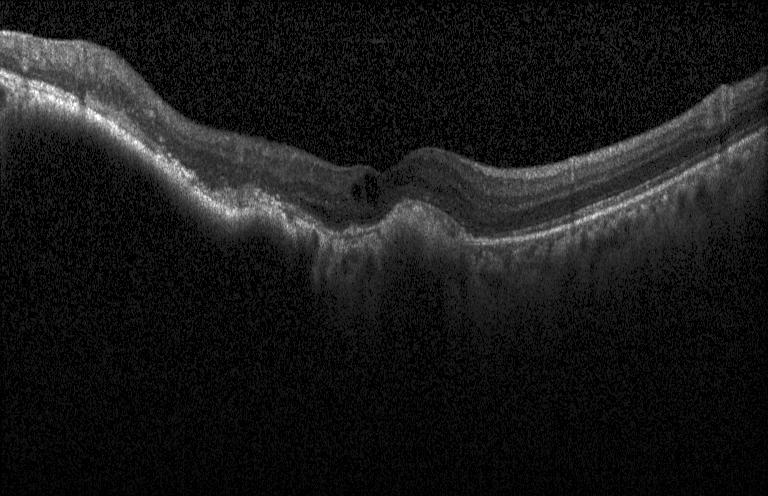 Acquired on a Heidelberg Spectralis, fovea-centered, spectral-domain OCT, retinal OCT cross-section
Assessment: choroidal neovascularization.